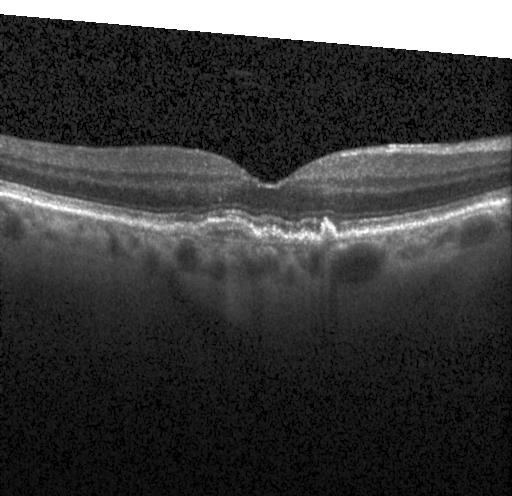 Spectral-domain OCT B-scan: a choroidal neovascular membrane.